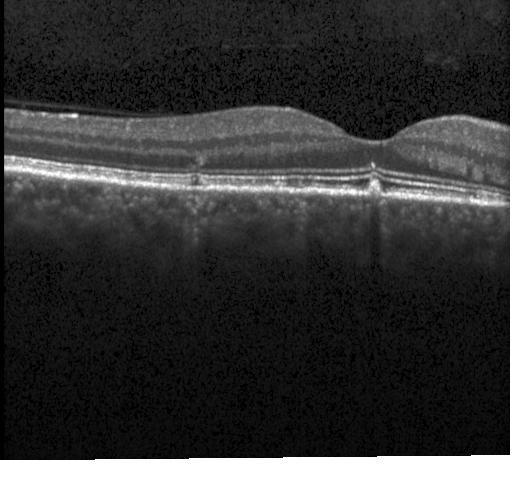 Retinal OCT cross-section.
Finding: sub-RPE drusenoid deposits.